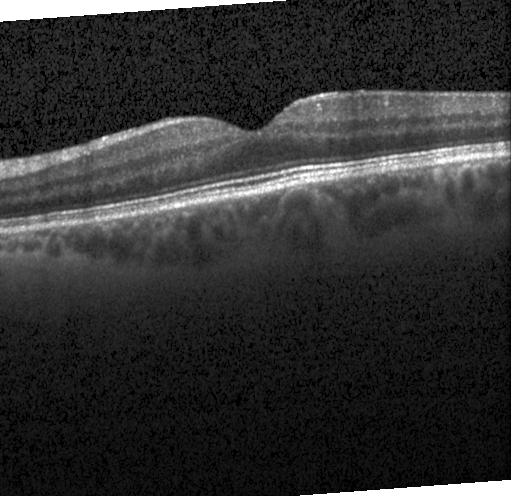
OCT line scan
The scan shows no evidence of choroidal neovascularization, diabetic macular edema, or drusen.